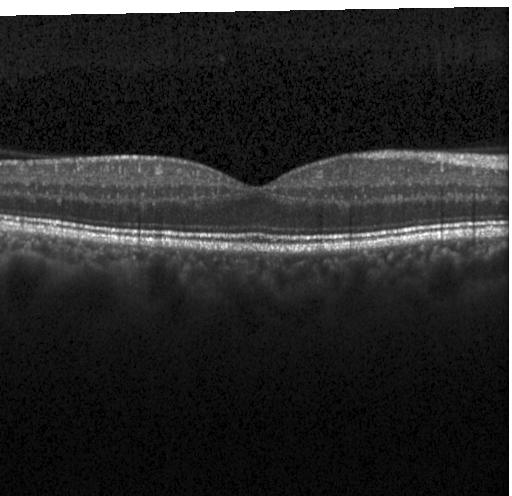

Dx: no choroidal neovascularization, no diabetic macular edema, and no drusen.